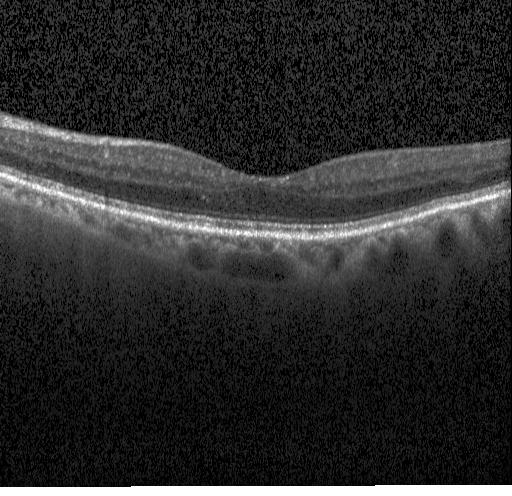 Macular OCT: neither CNV, DME, nor drusen.